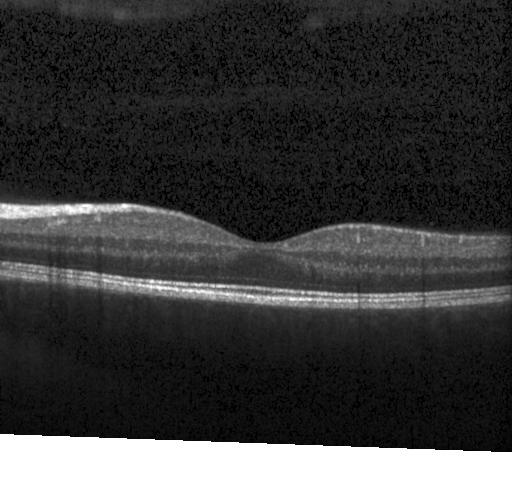

Macular scan · optical coherence tomography scan · spectral-domain optical coherence tomography · Heidelberg Spectralis OCT system
Finding: no choroidal neovascularization, no diabetic macular edema, and no drusen.